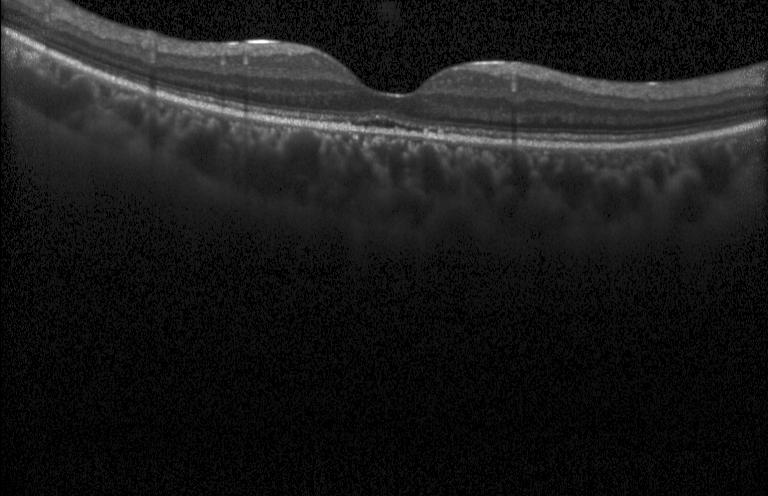 OCT B-scan. Heidelberg Spectralis. Spectral-domain optical coherence tomography
Diagnosis: no evidence of choroidal neovascularization, diabetic macular edema, or drusen.